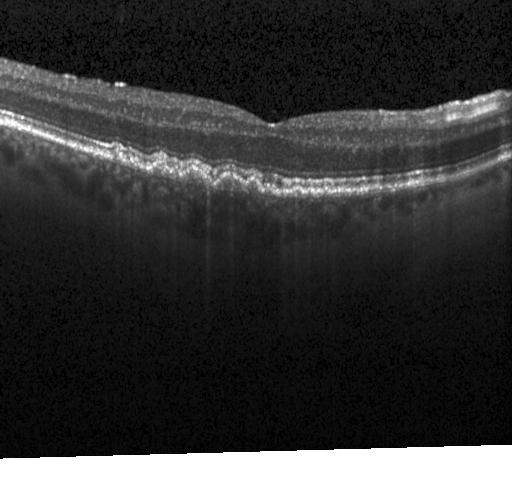
Spectral-domain optical coherence tomography, OCT B-scan. OCT finding: sub-RPE drusenoid deposits.